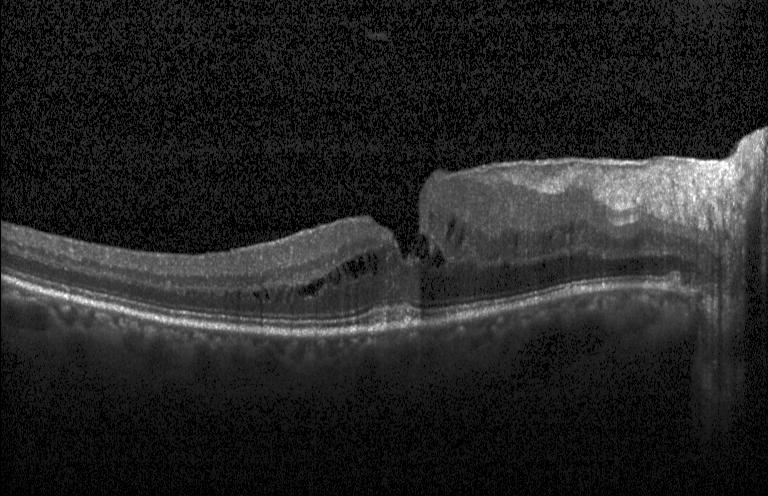 Macular scan. Instrument: Heidelberg Spectralis. Optical coherence tomography scan. SD-OCT.
Impression: DME.